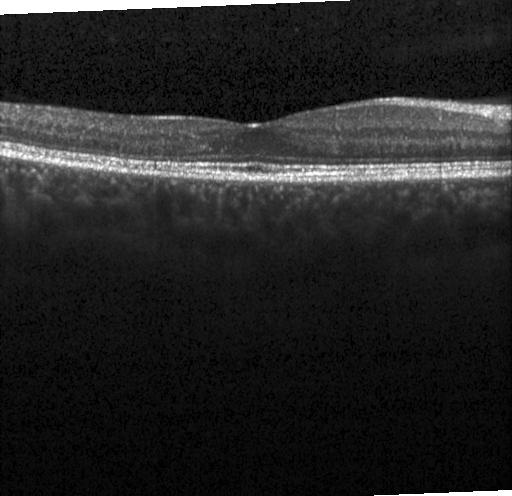

OCT line scan · spectral-domain OCT · horizontal scan through the fovea. Impression: no evidence of CNV, DME, or drusen.